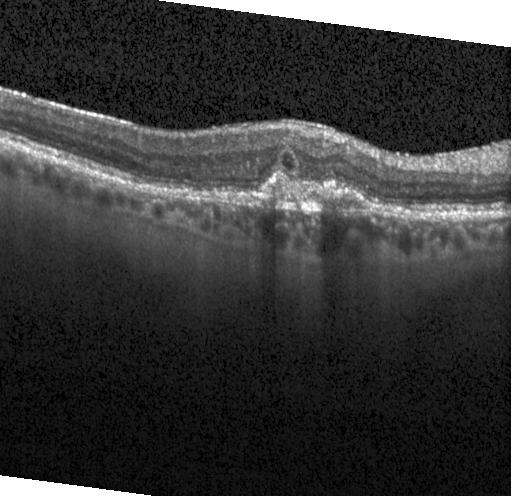

Diagnosis: choroidal neovascularization (CNV).